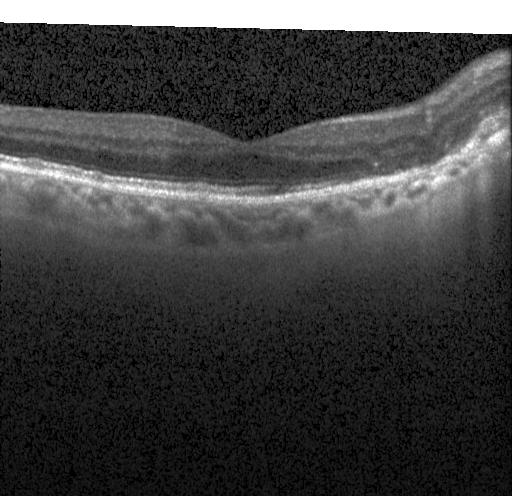 Acquired on a Heidelberg Spectralis · optical coherence tomography B-scan. Diagnosis: CNV.